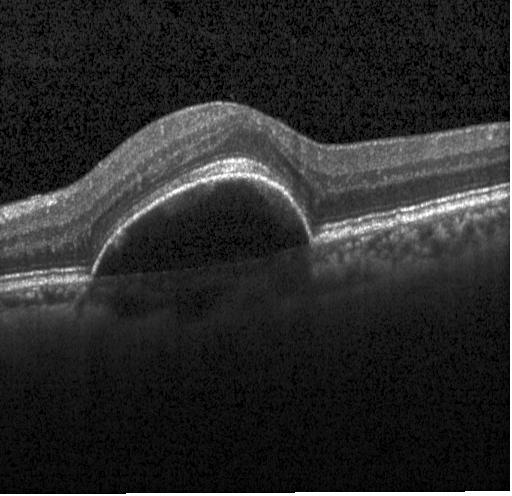

OCT B-scan showing a choroidal neovascular membrane.